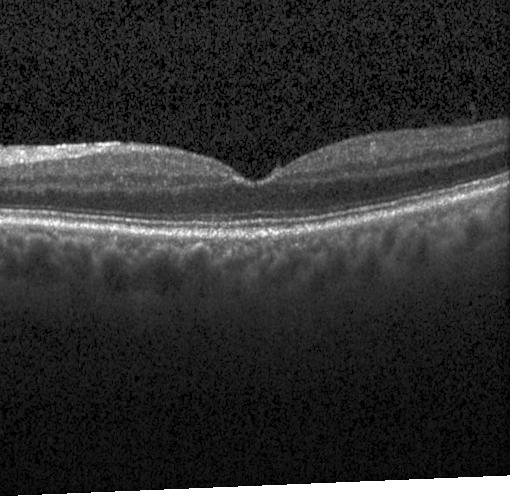 Impression: no choroidal neovascularization, no diabetic macular edema, and no drusen.